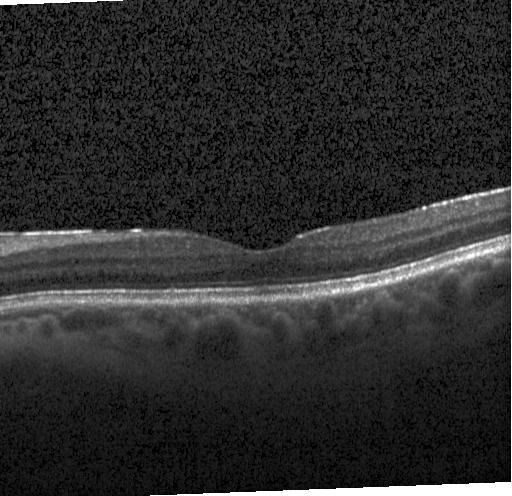

Spectral-domain OCT B-scan: neither choroidal neovascularization, diabetic macular edema, nor drusen.